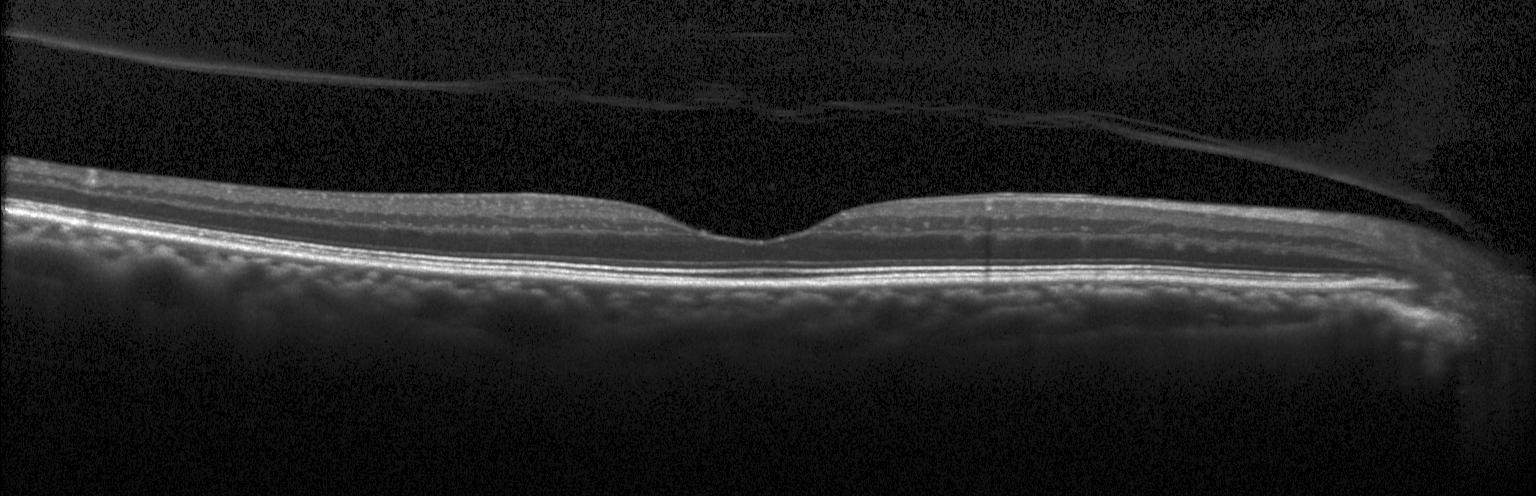

Optical coherence tomography B-scan — Impression: no evidence of CNV, DME, or drusen.